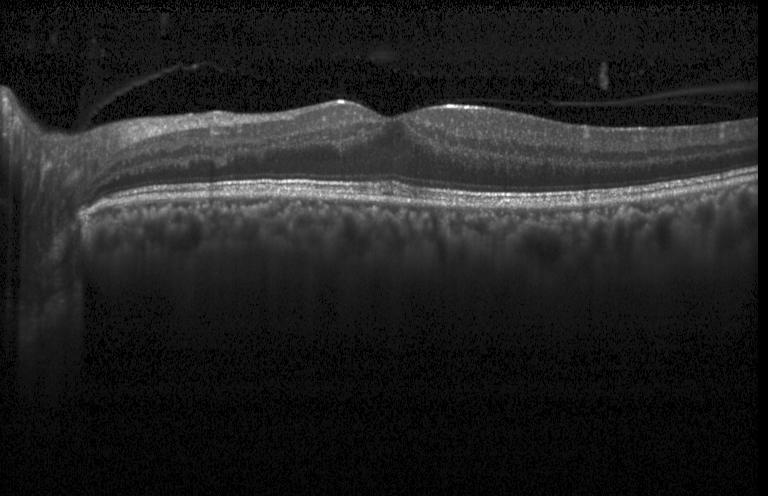 Spectral-domain OCT; macular scan; Heidelberg Spectralis OCT system; optical coherence tomography B-scan. Finding: no choroidal neovascularization, diabetic macular edema, or drusen.